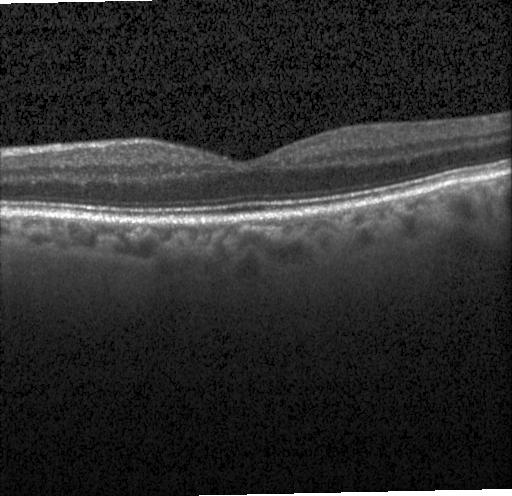

Diagnosis: no evidence of CNV, DME, or drusen.